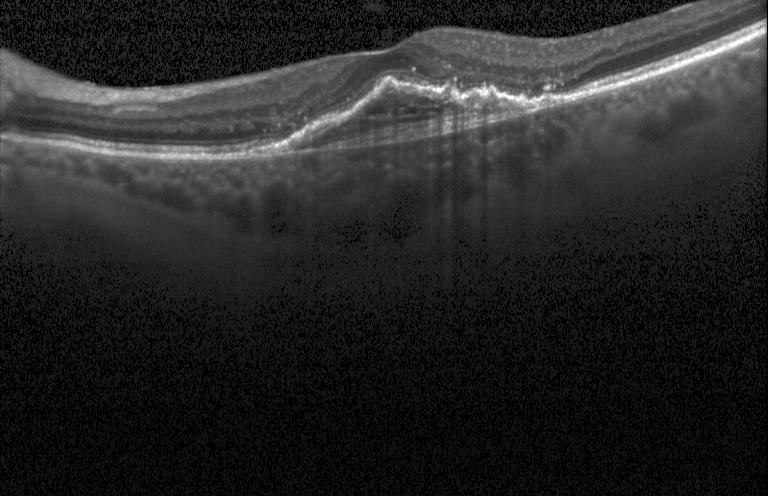 Finding: a choroidal neovascular membrane.